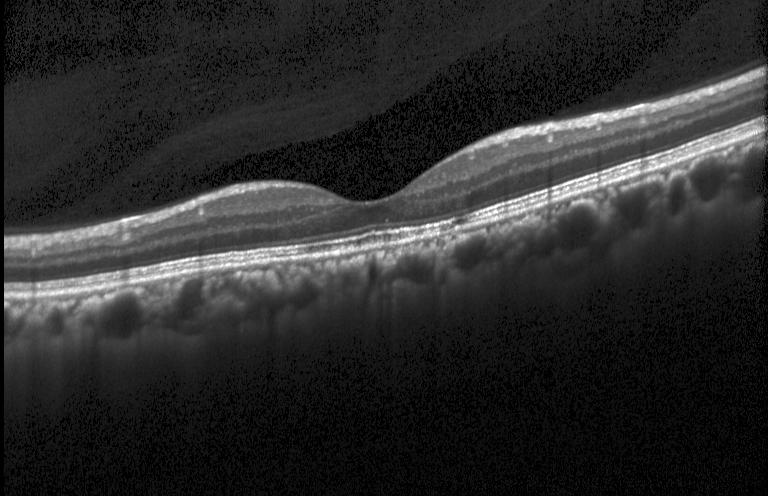 Spectral-domain OCT B-scan: no choroidal neovascularization, diabetic macular edema, or drusen.